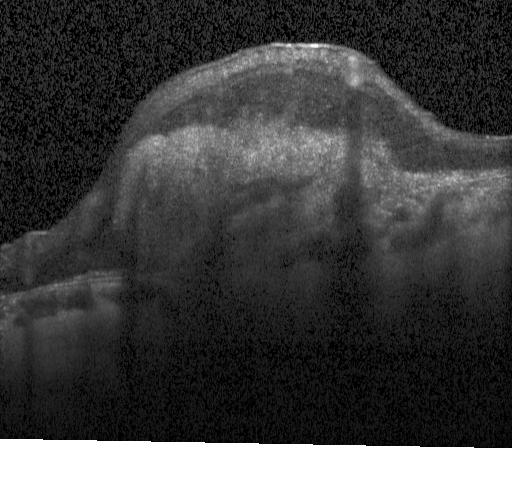 Optical coherence tomography B-scan, horizontal scan through the fovea, Heidelberg Spectralis, spectral-domain OCT. Dx: a choroidal neovascular membrane.